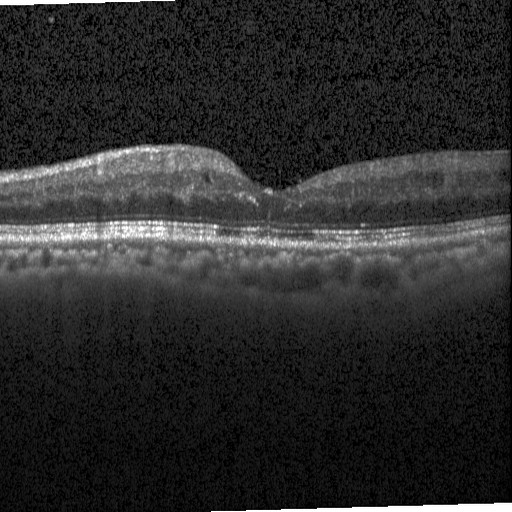 Optical coherence tomography scan; Heidelberg Spectralis OCT system; horizontal scan through the fovea.
This B-scan demonstrates DME.